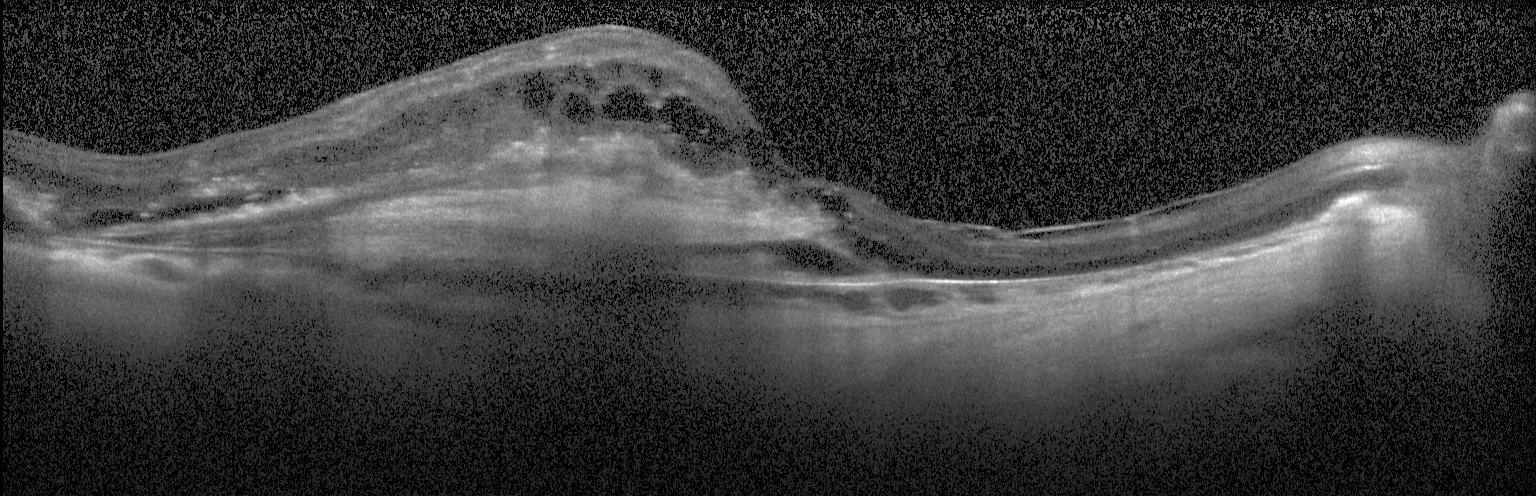 OCT B-scan.
Finding: a choroidal neovascular membrane.